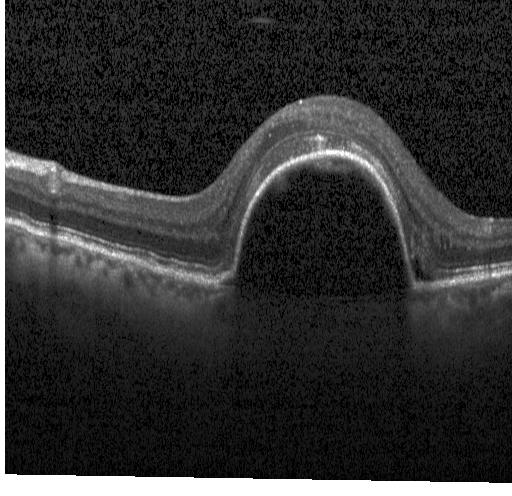
OCT line scan
The scan shows a choroidal neovascular membrane.